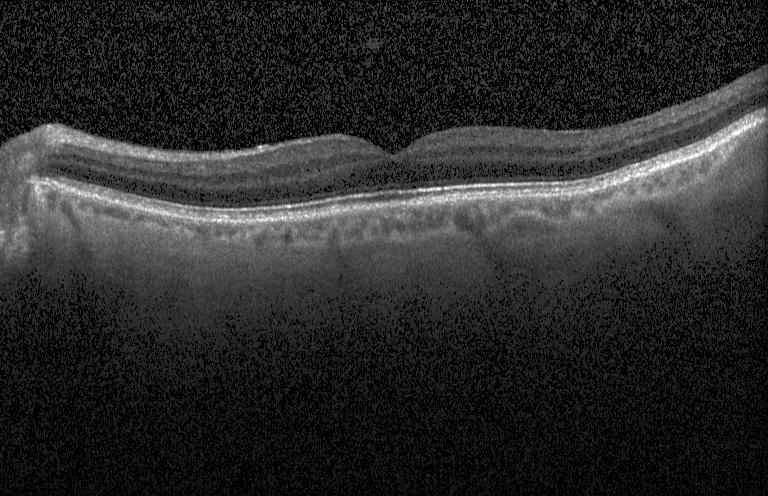 Retinal OCT cross-section — Finding: no choroidal neovascularization, diabetic macular edema, or drusen.